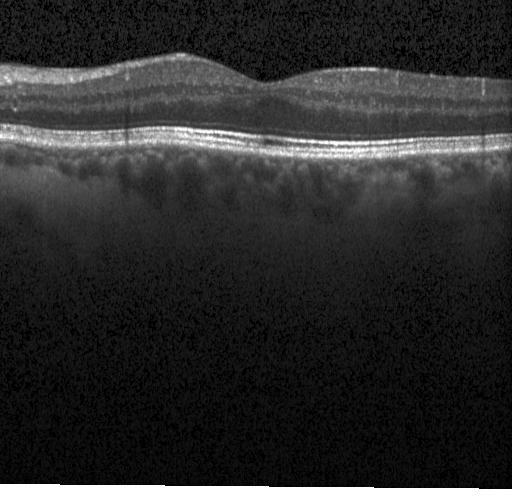

Through the macula; optical coherence tomography B-scan. Finding: no choroidal neovascularization, diabetic macular edema, or drusen.